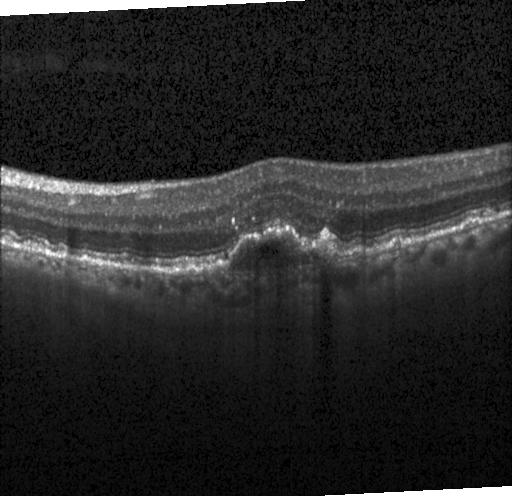

Optical coherence tomography B-scan; spectral-domain optical coherence tomography; centered on the fovea
A choroidal neovascular membrane.